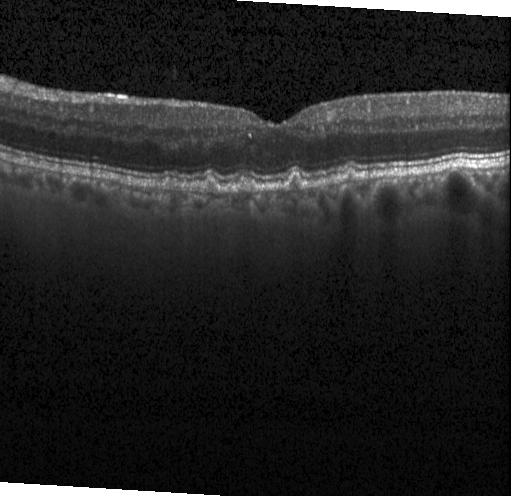
OCT line scan — The scan shows sub-RPE drusenoid deposits.